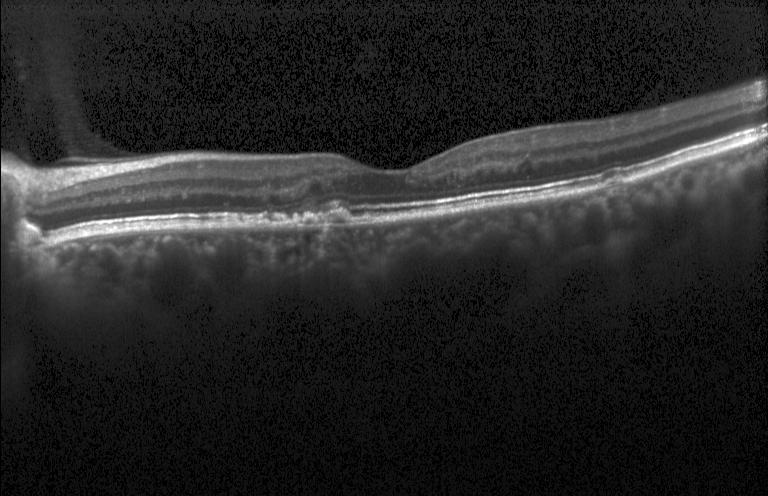 This B-scan demonstrates CNV.